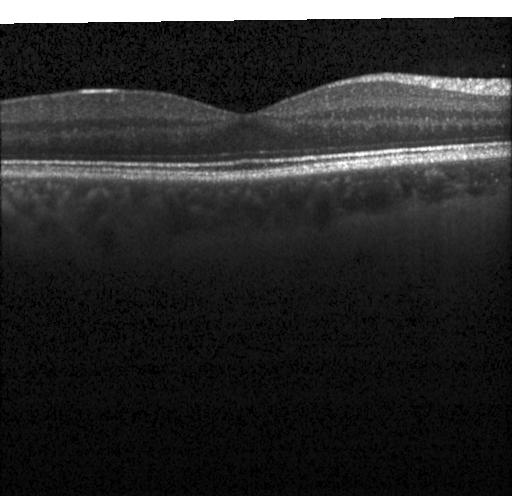

Spectral-domain optical coherence tomography, optical coherence tomography scan, fovea-centered, acquired on a Heidelberg Spectralis.
Impression: neither choroidal neovascularization, diabetic macular edema, nor drusen.